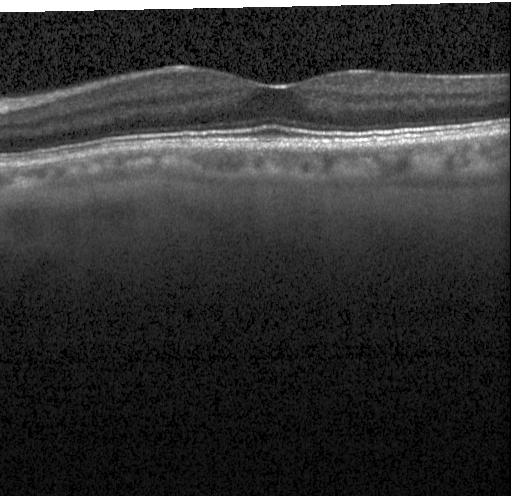

Heidelberg Spectralis; retinal OCT cross-section
Impression: neither CNV, DME, nor drusen.